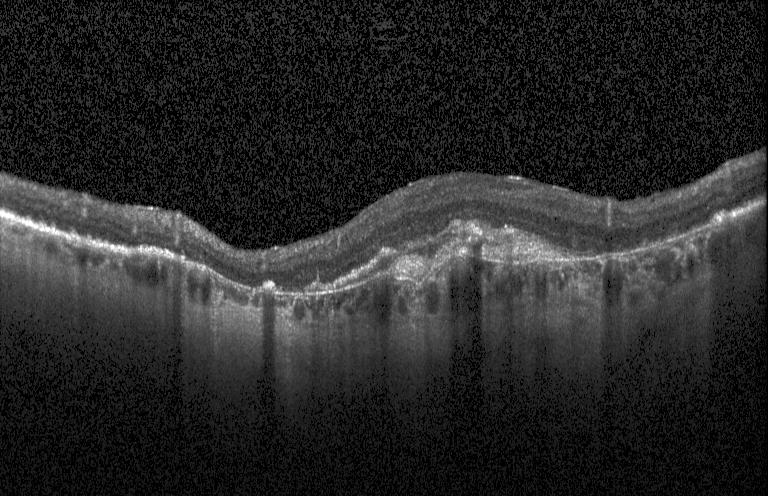 Retinal OCT B-scan; spectral-domain OCT — Impression: CNV.